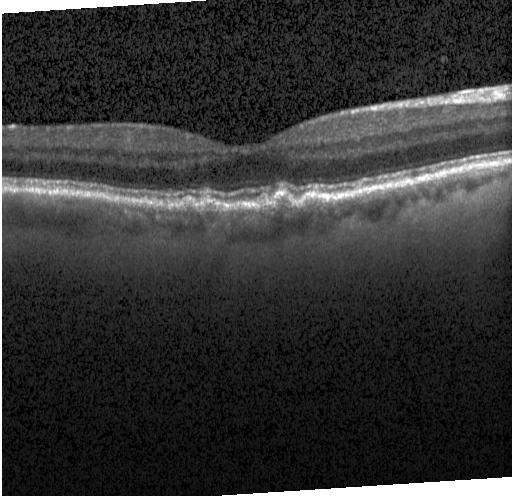

Horizontal scan through the fovea. Retinal OCT B-scan.
Diagnosis: sub-RPE drusenoid deposits.